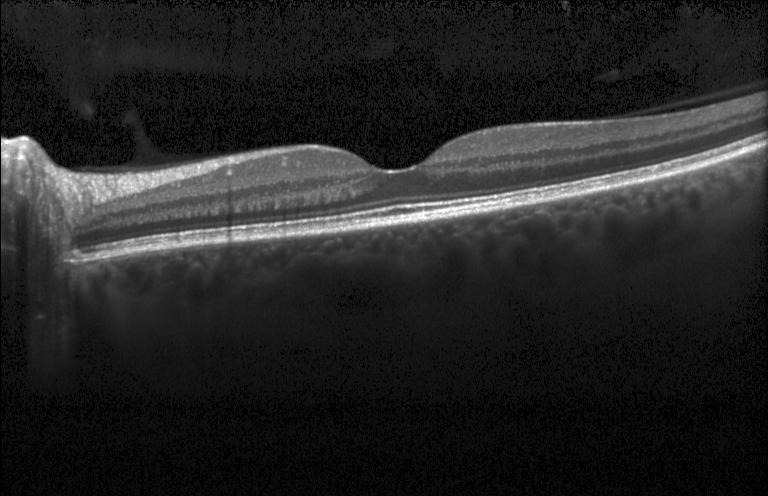
OCT line scan. Diagnosis: no choroidal neovascularization, no diabetic macular edema, and no drusen.